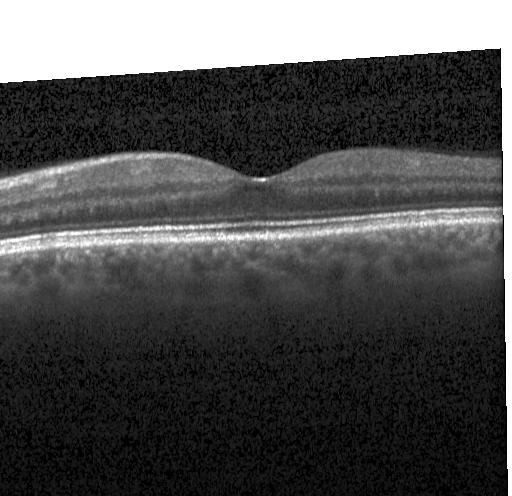

Diagnosis: no choroidal neovascularization, no diabetic macular edema, and no drusen.